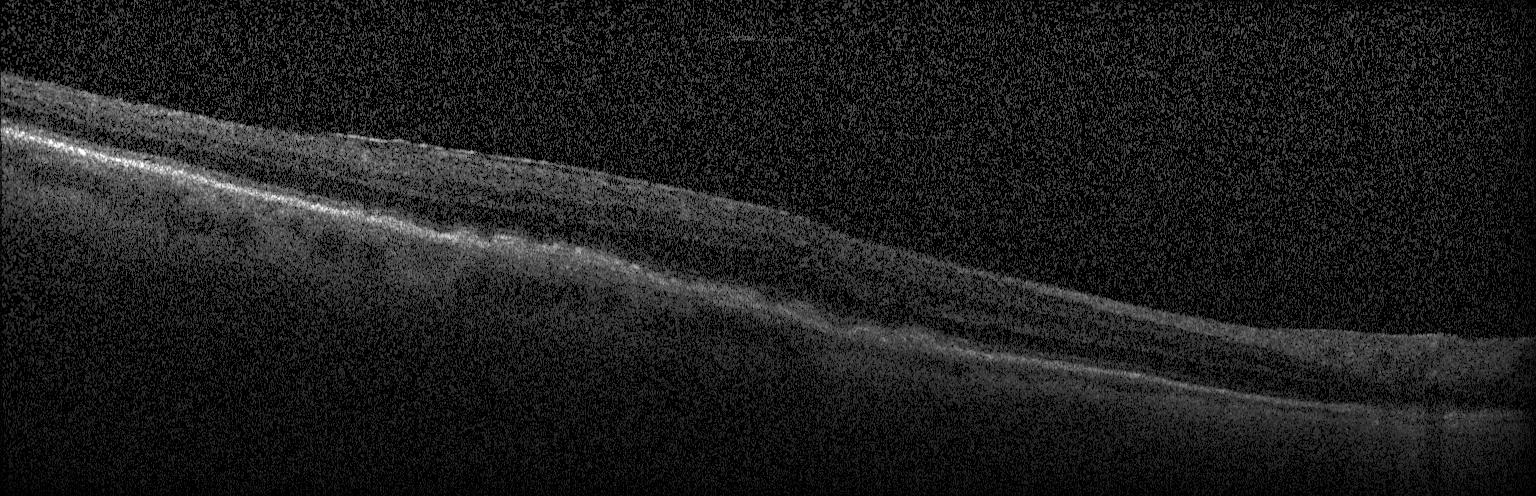

OCT line scan
Finding: multiple drusen.